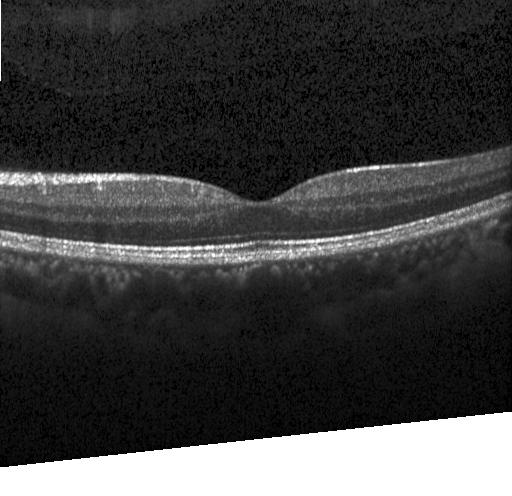 Heidelberg Spectralis · optical coherence tomography scan
Impression: no evidence of CNV, DME, or drusen.